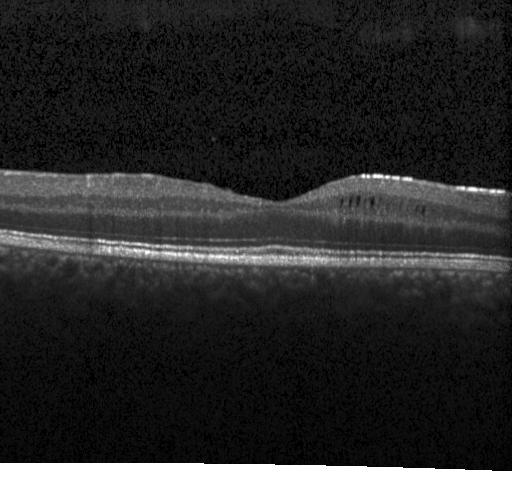

Assessment: DME.